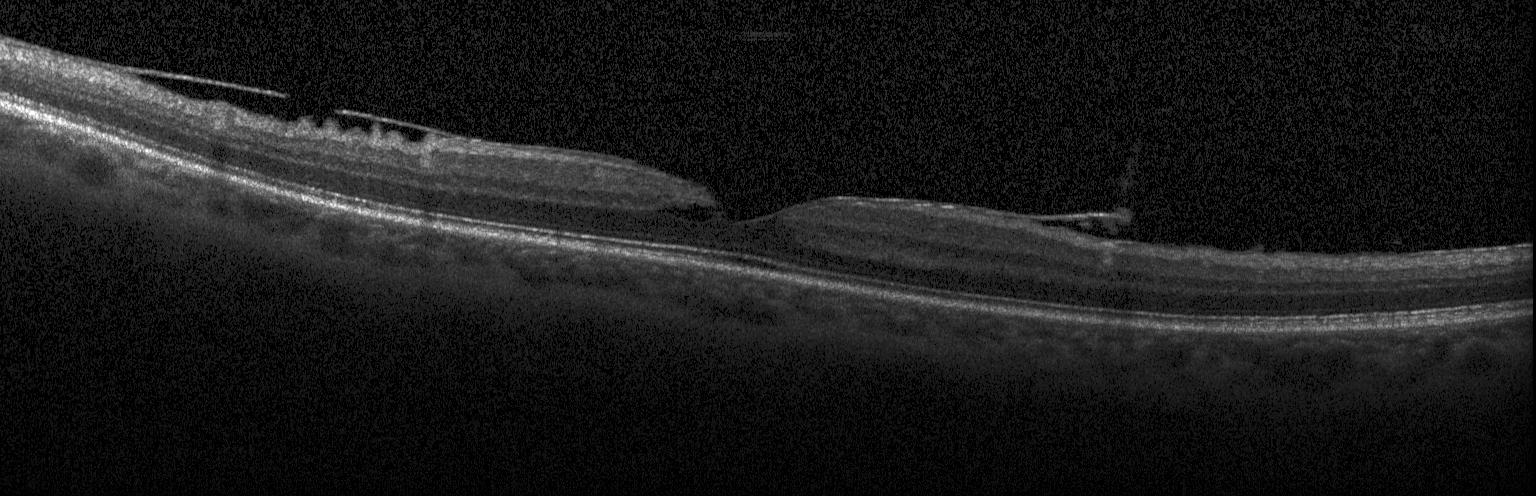 Optical coherence tomography scan; SD-OCT; macular scan.
The scan shows diabetic macular edema (DME).